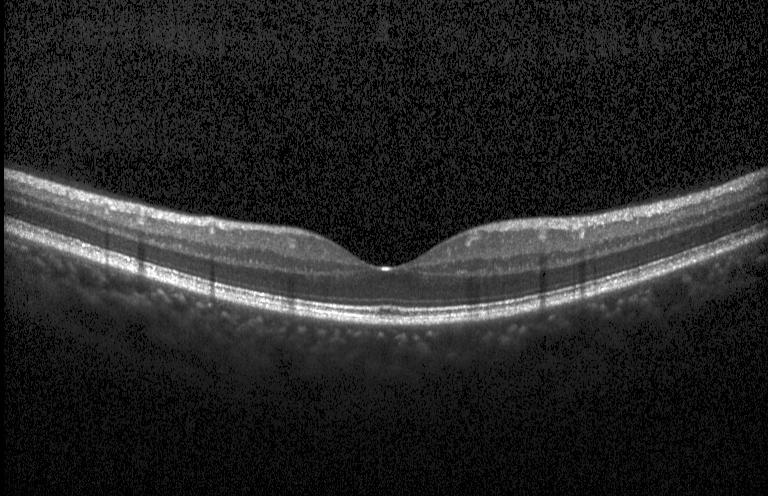 Spectral-domain OCT, retinal OCT B-scan. Finding: no choroidal neovascularization, no diabetic macular edema, and no drusen.